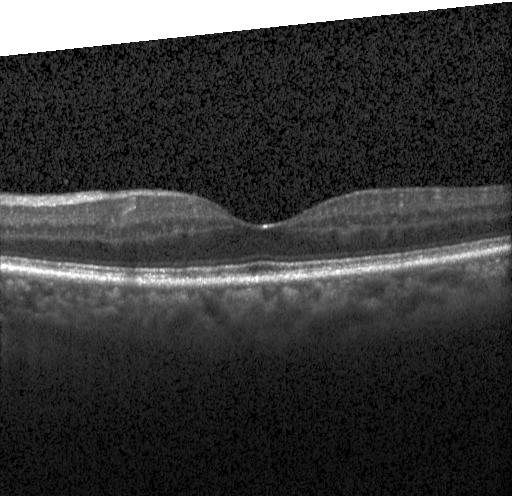
OCT finding: no choroidal neovascularization, no diabetic macular edema, and no drusen.